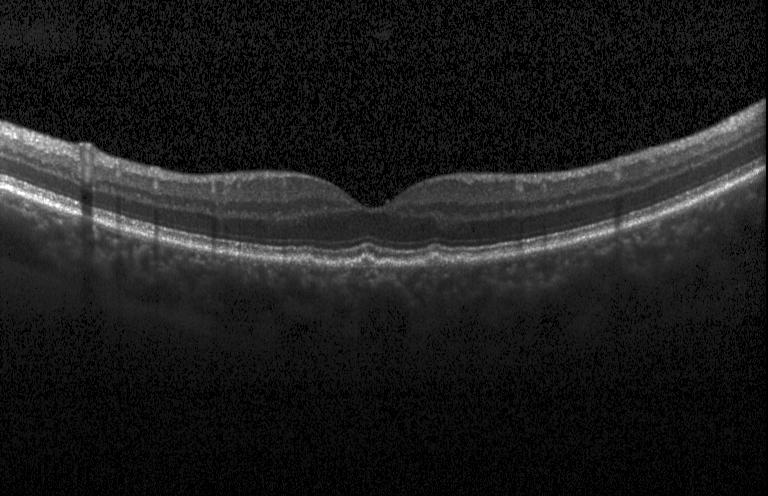

Diagnosis: multiple drusen.